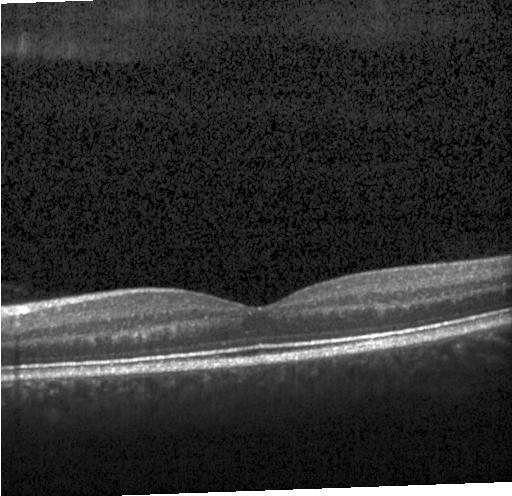

Macular OCT: no choroidal neovascularization, diabetic macular edema, or drusen.